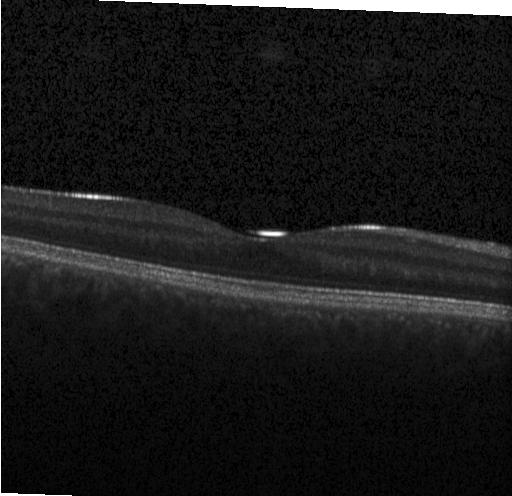 Impression: no evidence of CNV, DME, or drusen.